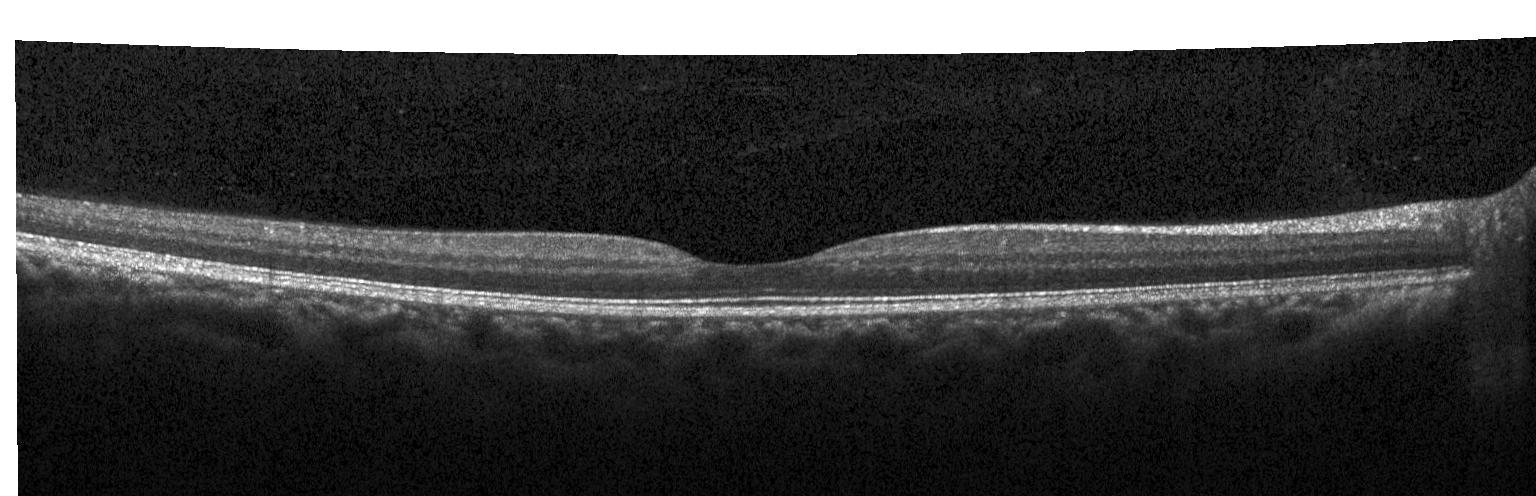 Heidelberg Spectralis. OCT B-scan — Macular OCT: no choroidal neovascularization, diabetic macular edema, or drusen.